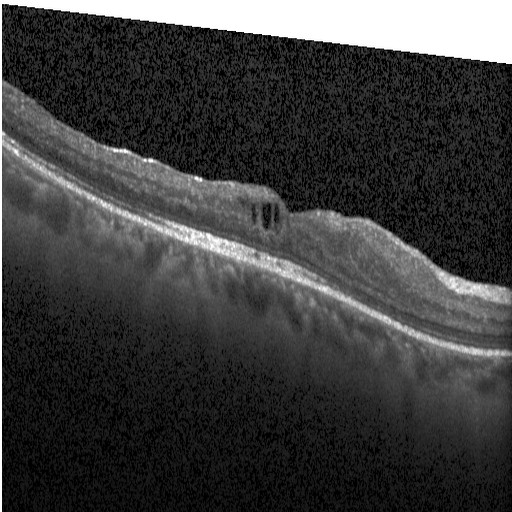 OCT scan showing DME.